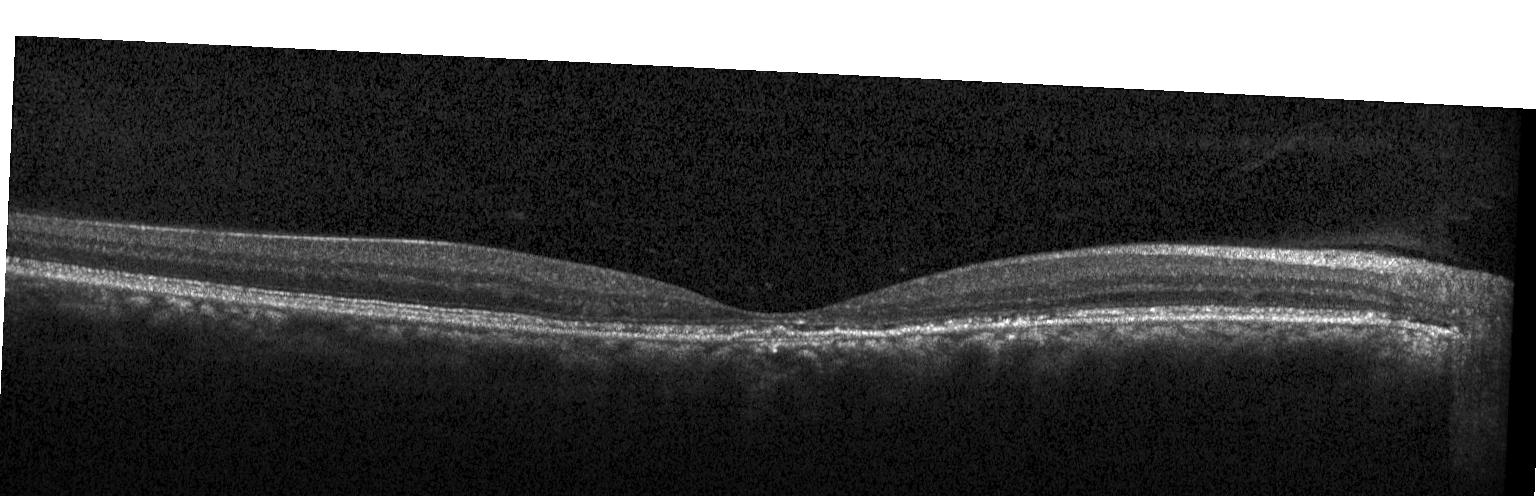
Optical coherence tomography B-scan — A choroidal neovascular membrane.